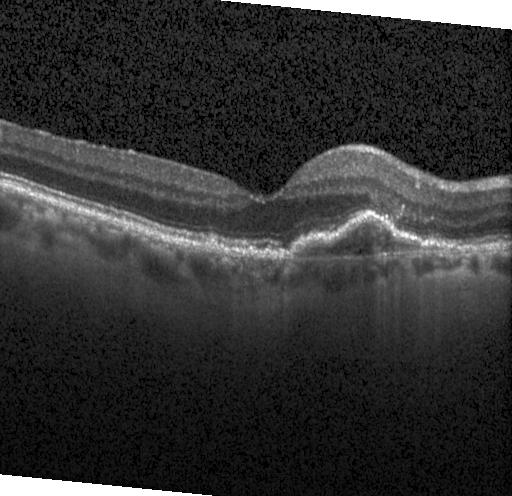 Spectral-domain optical coherence tomography; instrument: Heidelberg Spectralis; optical coherence tomography B-scan — Diagnosis: a choroidal neovascular membrane.